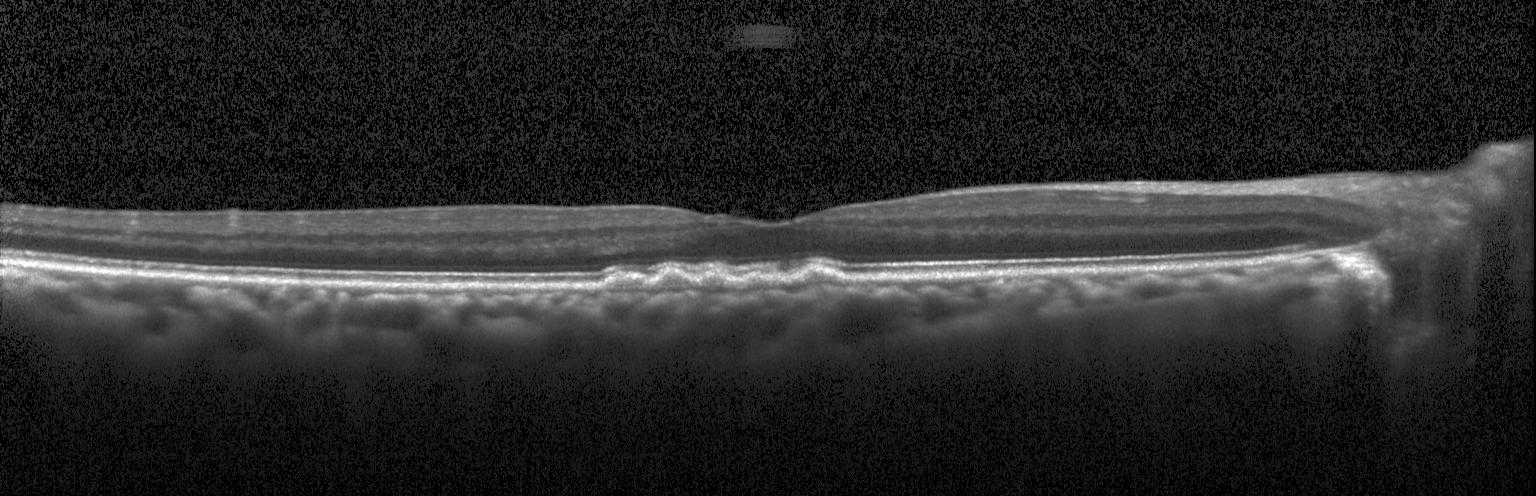
Optical coherence tomography B-scan. Finding: multiple drusen.